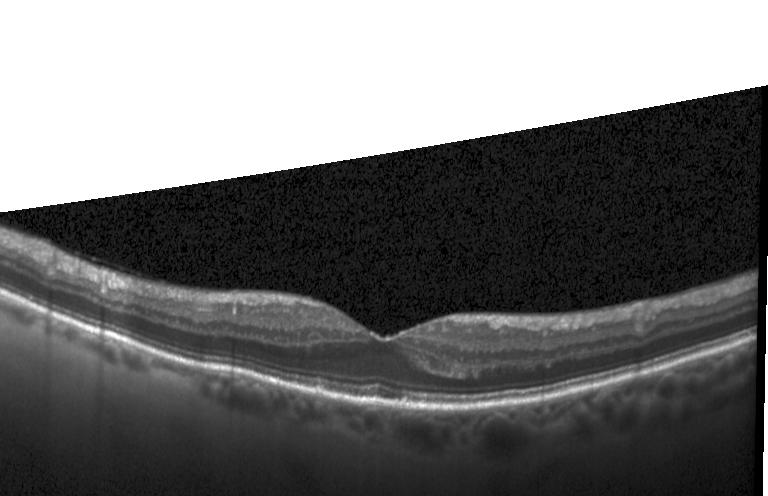
Optical coherence tomography scan
Finding: no choroidal neovascularization, no diabetic macular edema, and no drusen.